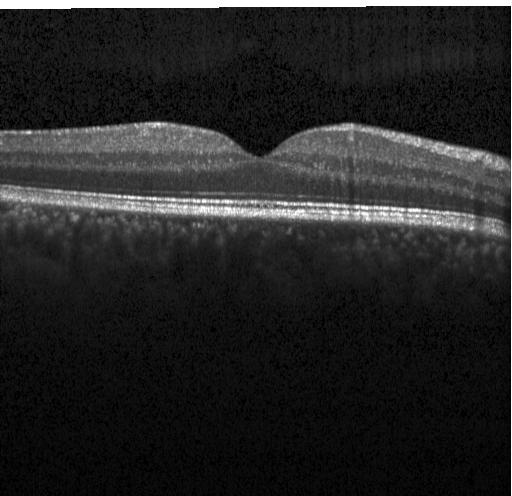
Optical coherence tomography scan — Assessment: no choroidal neovascularization, no diabetic macular edema, and no drusen.